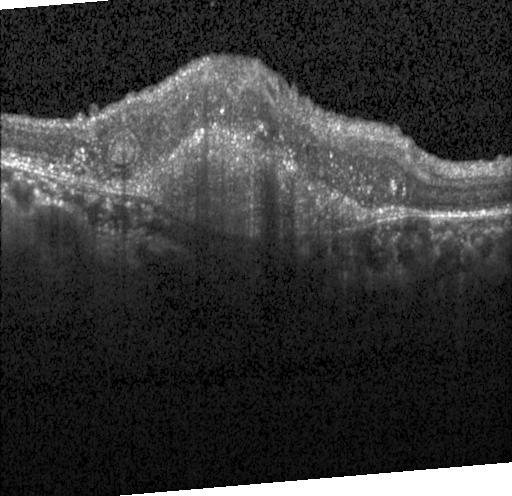
Finding: a choroidal neovascular membrane.